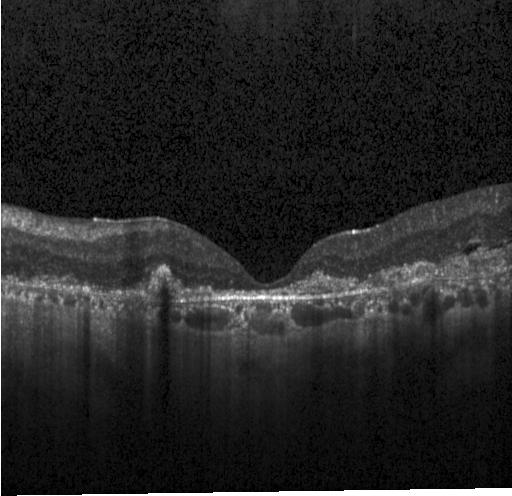

Impression: a choroidal neovascular membrane.